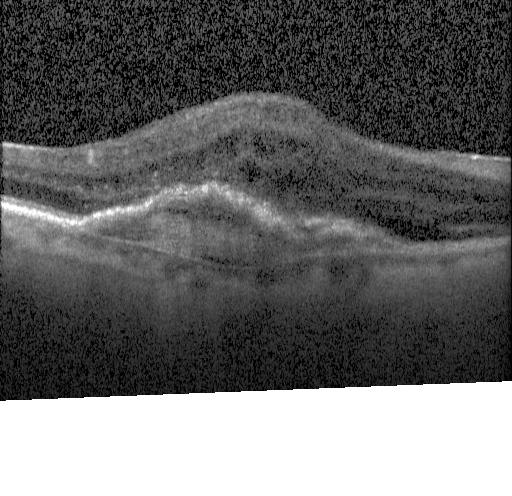

Spectral-domain optical coherence tomography; retinal OCT cross-section; Heidelberg Spectralis OCT system; fovea-centered — Diagnosis: a choroidal neovascular membrane.